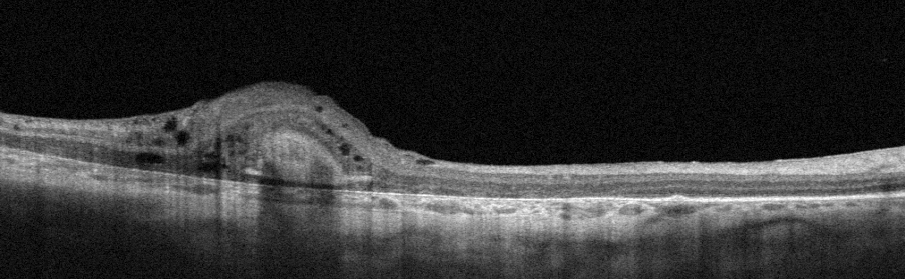
Retinal OCT B-scan. Impression: age-related macular degeneration.